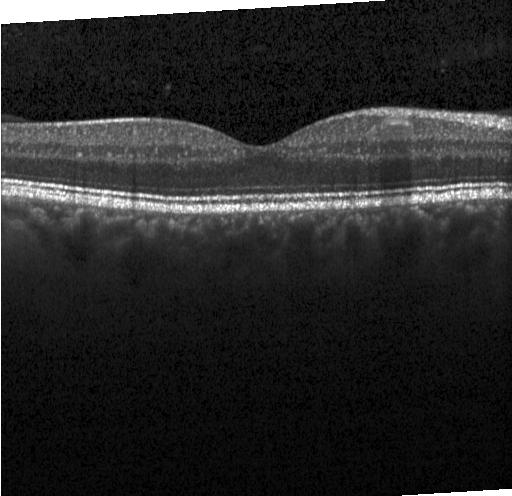

Retinal OCT B-scan.
No choroidal neovascularization, no diabetic macular edema, and no drusen.